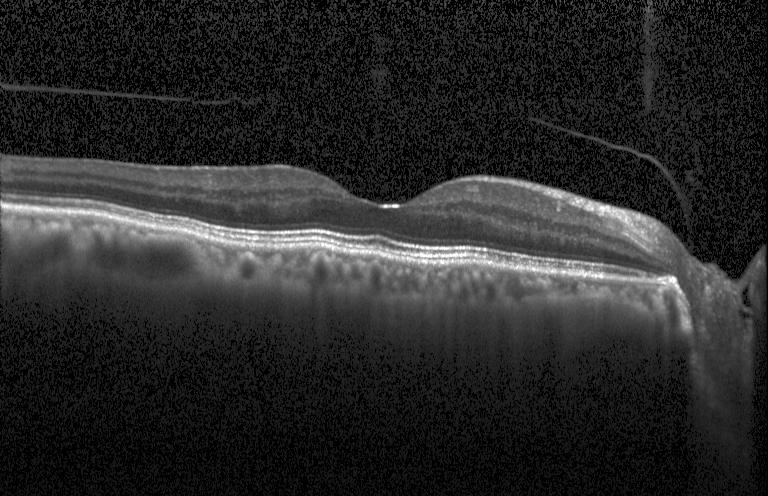
Macular OCT demonstrating no choroidal neovascularization, diabetic macular edema, or drusen.